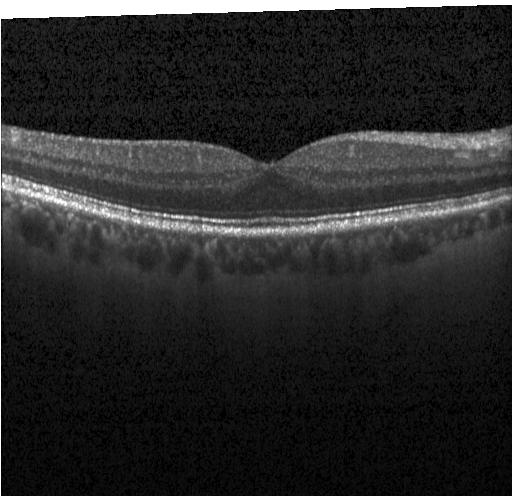
OCT line scan. Instrument: Heidelberg Spectralis. Spectral-domain optical coherence tomography.
Impression: neither choroidal neovascularization, diabetic macular edema, nor drusen.